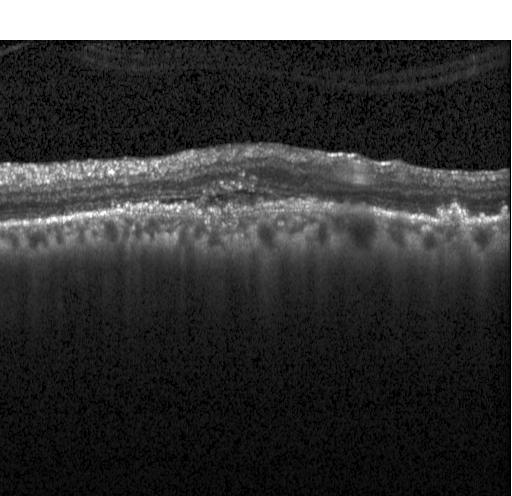 Retinal OCT cross-section showing a choroidal neovascular membrane.